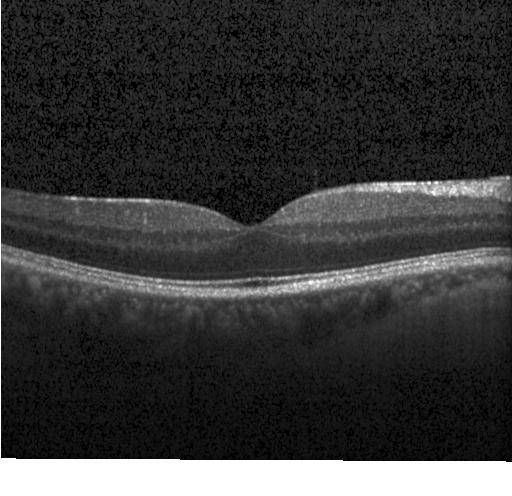

Optical coherence tomography B-scan
No choroidal neovascularization, no diabetic macular edema, and no drusen.